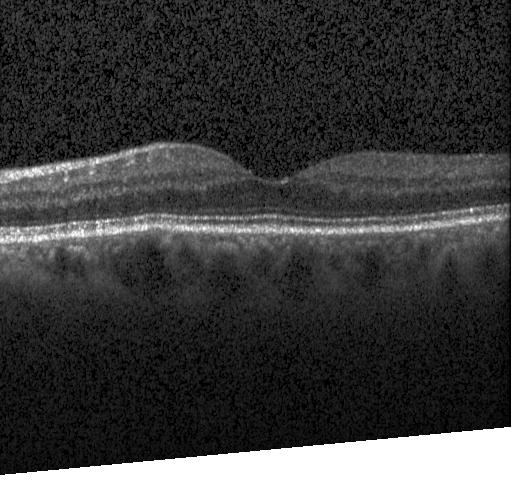
Impression: no evidence of choroidal neovascularization, diabetic macular edema, or drusen.